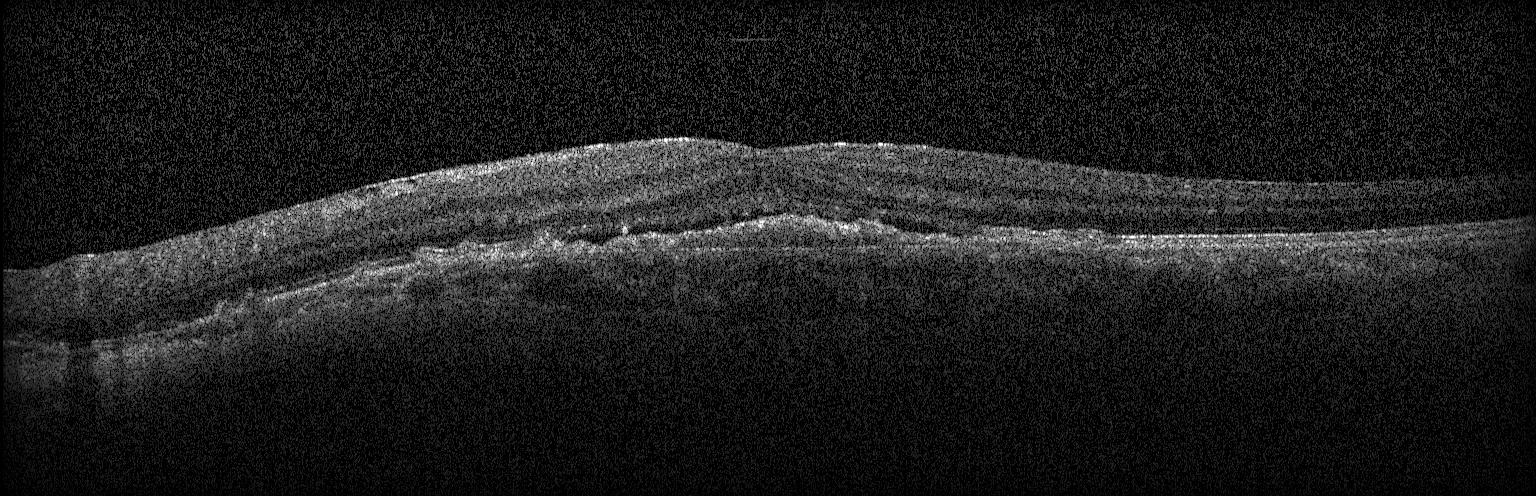 Optical coherence tomography scan · horizontal scan through the fovea — The scan shows a choroidal neovascular membrane.